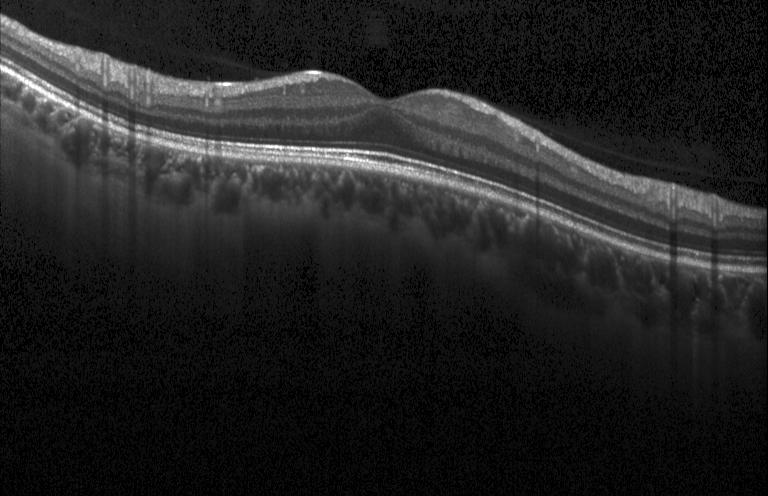
Finding: no CNV, no DME, and no drusen.